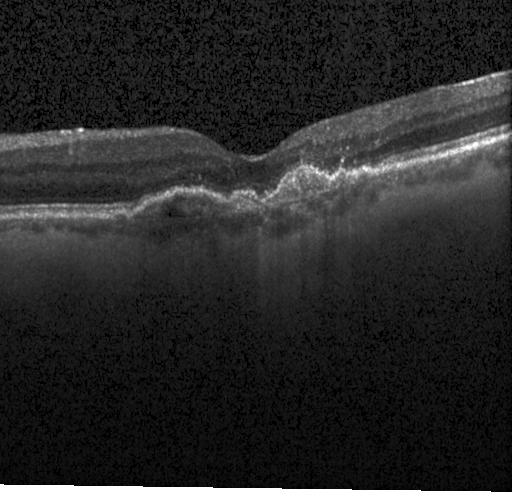 Optical coherence tomography B-scan.
Diagnosis: choroidal neovascularization.